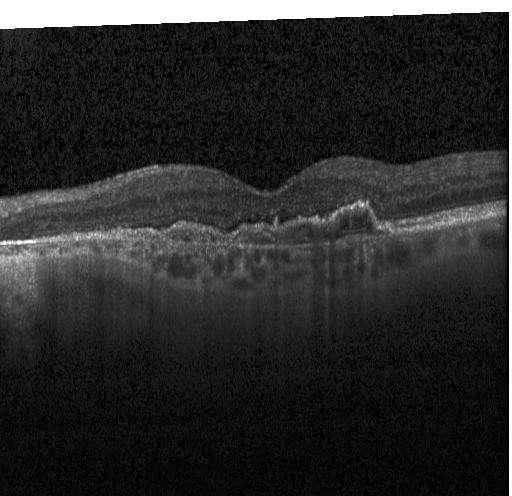
This B-scan demonstrates CNV.